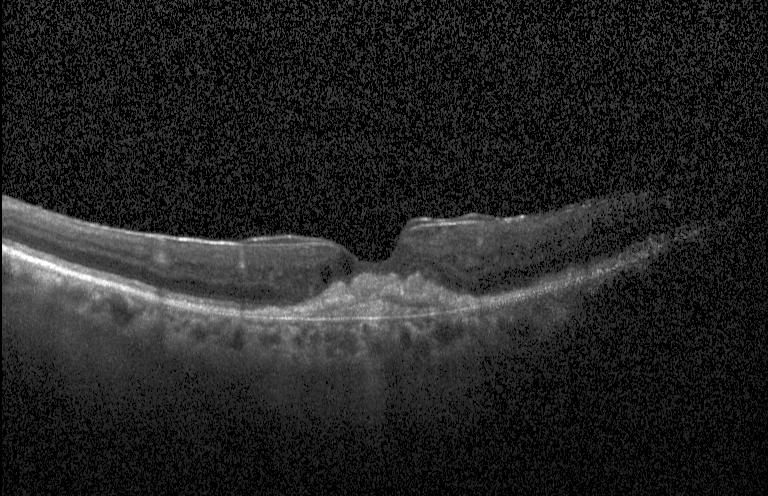

Assessment: a choroidal neovascular membrane.